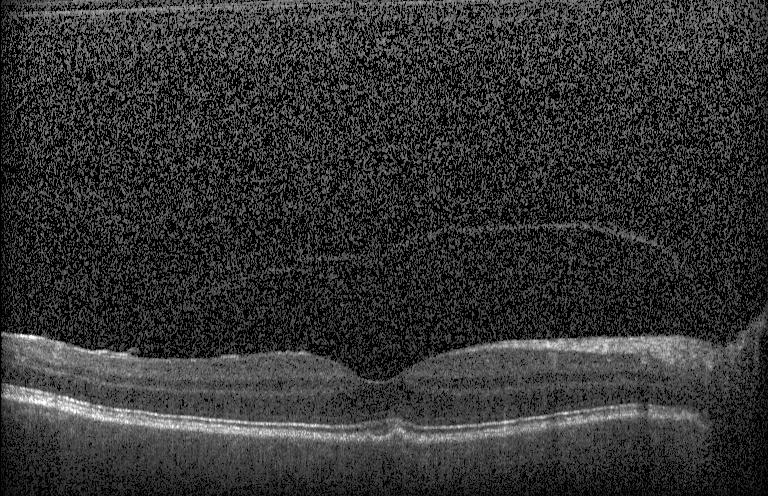
OCT B-scan; SD-OCT.
The scan shows sub-RPE drusenoid deposits.